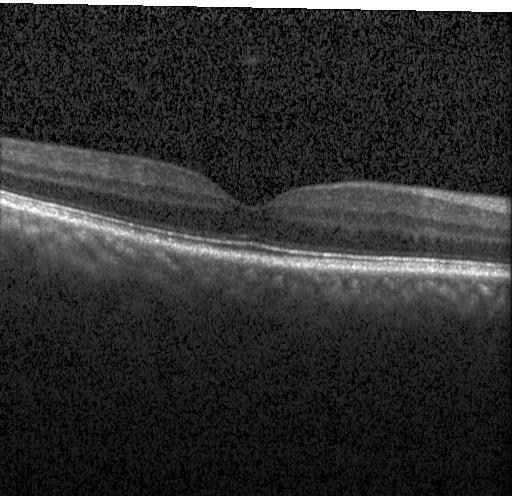
OCT B-scan; spectral-domain optical coherence tomography; instrument: Heidelberg Spectralis; macular scan. Finding: neither CNV, DME, nor drusen.